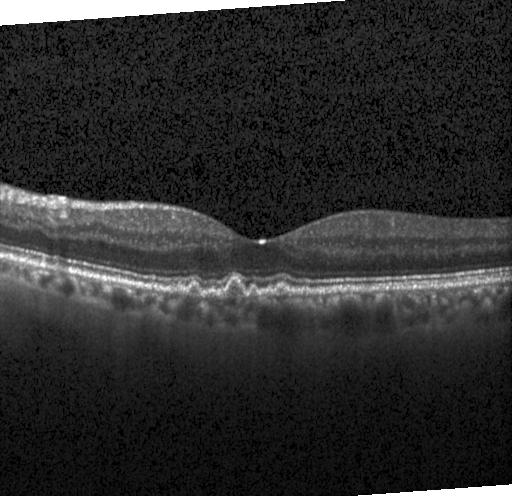

SD-OCT · Heidelberg Spectralis · horizontal scan through the fovea · optical coherence tomography scan
OCT finding: multiple drusen.